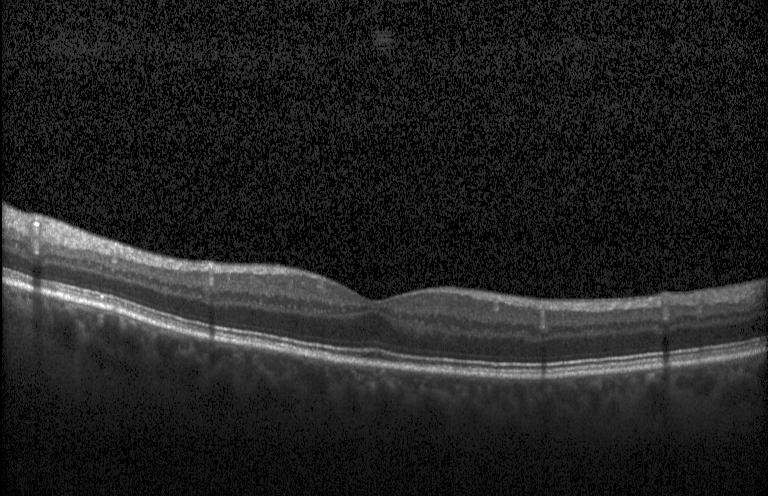
Optical coherence tomography scan, centered on the fovea, instrument: Heidelberg Spectralis.
Diagnosis: neither choroidal neovascularization, diabetic macular edema, nor drusen.